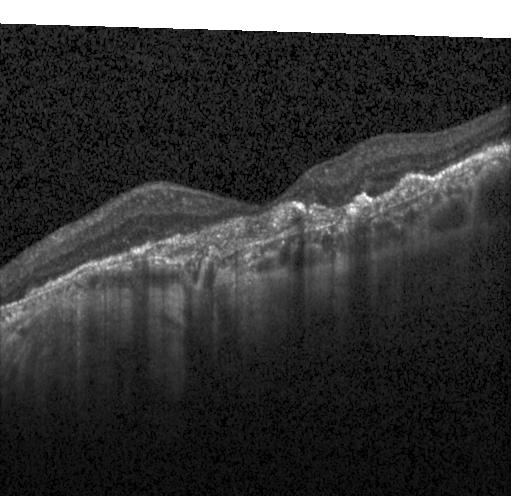
Diagnosis: a choroidal neovascular membrane.